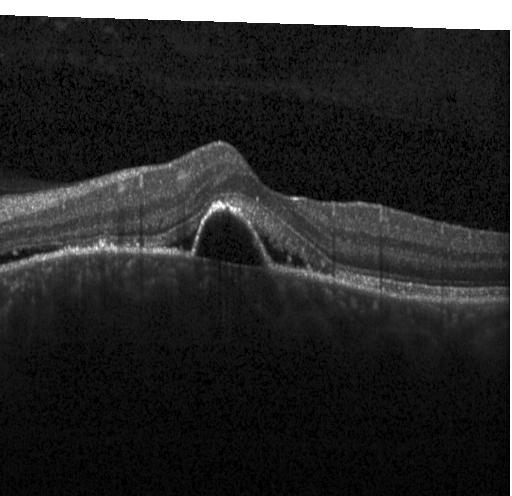

Diagnosis: a choroidal neovascular membrane.